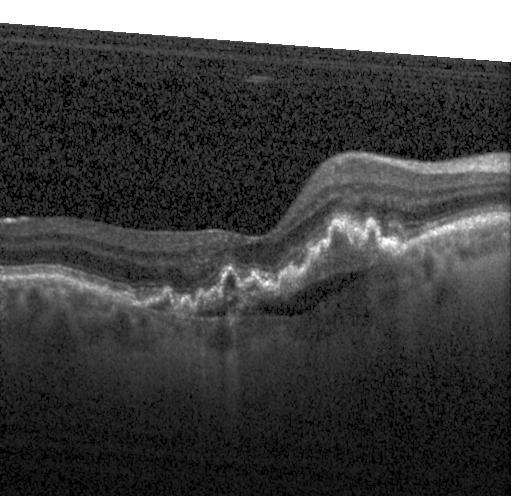
The scan shows a choroidal neovascular membrane.